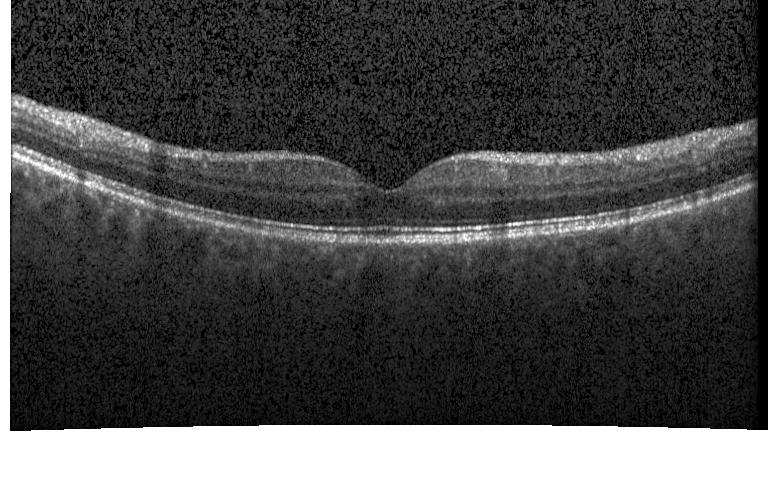
SD-OCT · instrument: Heidelberg Spectralis · retinal OCT cross-section · horizontal scan through the fovea.
This B-scan demonstrates no choroidal neovascularization, diabetic macular edema, or drusen.